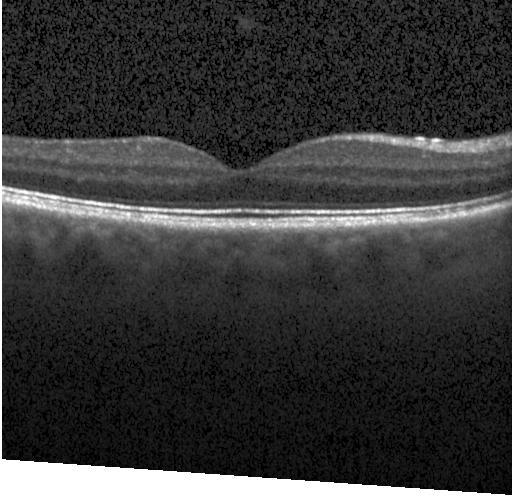
No choroidal neovascularization, no diabetic macular edema, and no drusen.